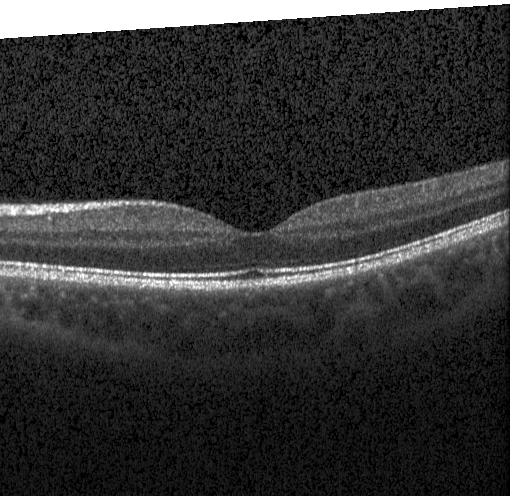 No choroidal neovascularization, no diabetic macular edema, and no drusen.